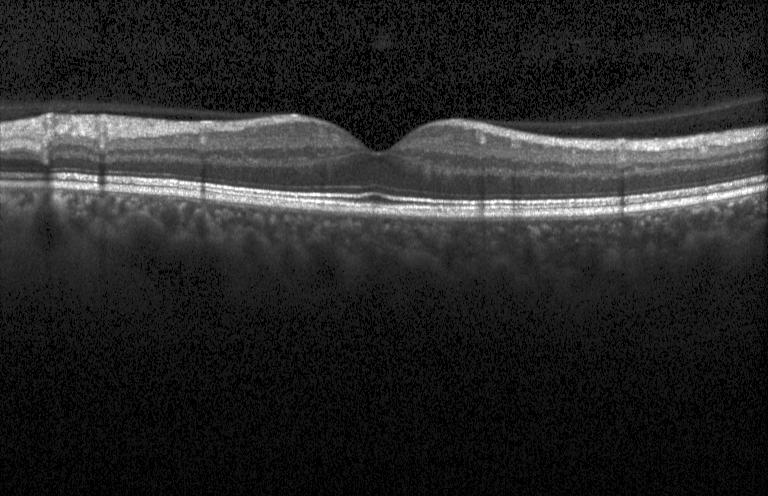

This B-scan demonstrates no CNV, DME, or drusen.